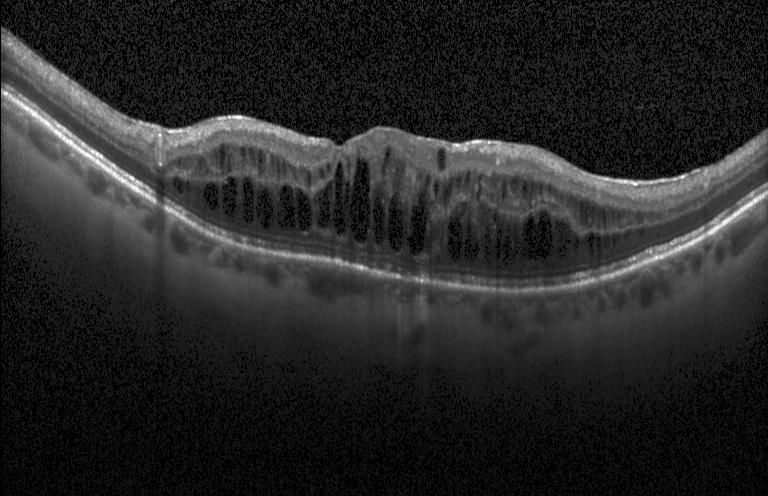
Impression: diabetic macular edema (DME).